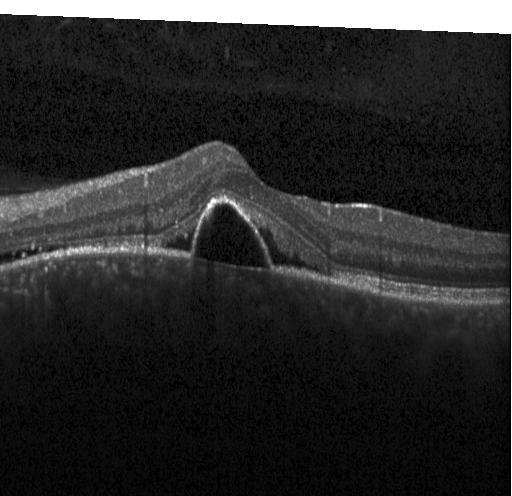 This B-scan demonstrates choroidal neovascularization.